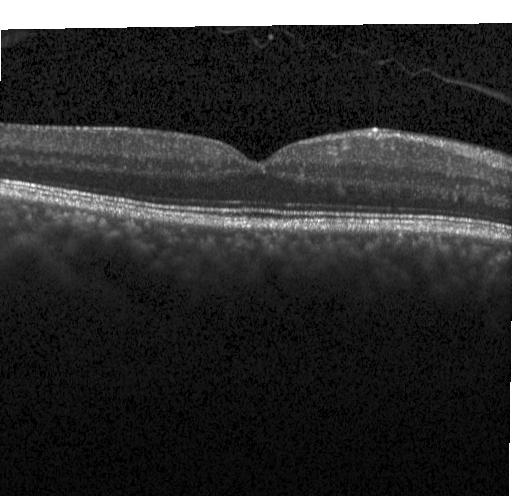 No evidence of choroidal neovascularization, diabetic macular edema, or drusen.